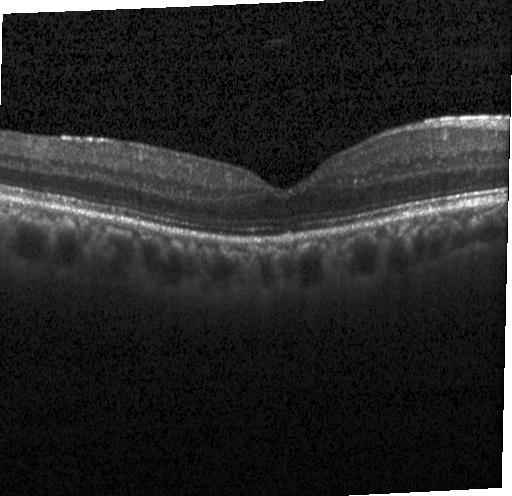

Dx: neither choroidal neovascularization, diabetic macular edema, nor drusen.